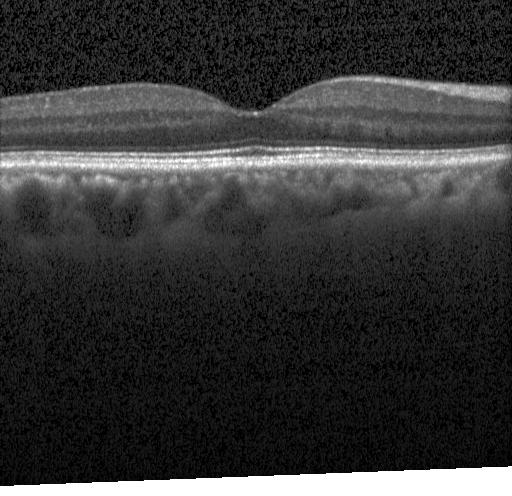

Optical coherence tomography scan — OCT finding: no evidence of CNV, DME, or drusen.